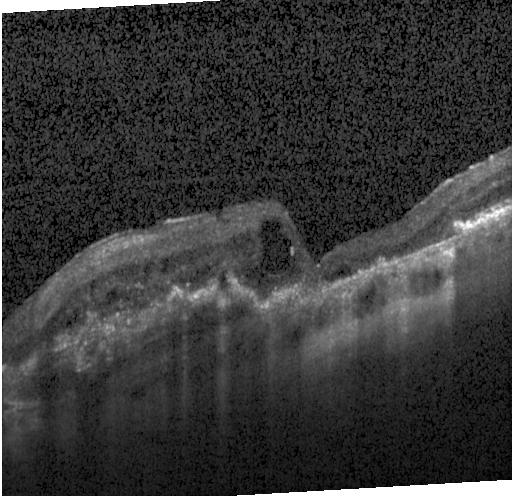
Spectral-domain optical coherence tomography. OCT B-scan. Acquired on a Heidelberg Spectralis.
Finding: choroidal neovascularization (CNV).